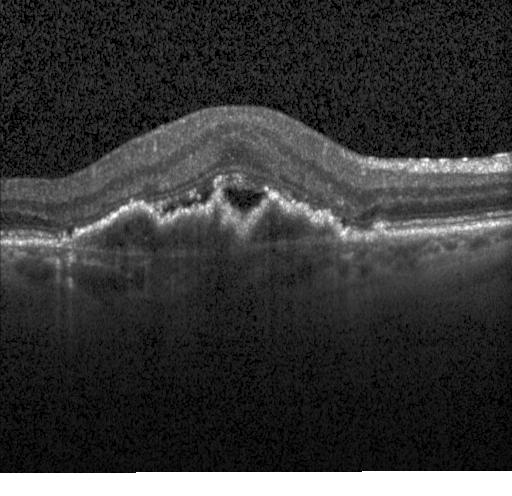
Spectral-domain OCT B-scan: choroidal neovascularization.